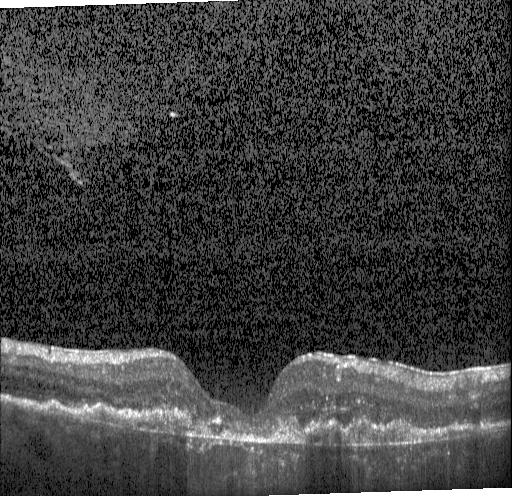 Instrument: Heidelberg Spectralis, spectral-domain OCT, OCT B-scan
Finding: CNV.